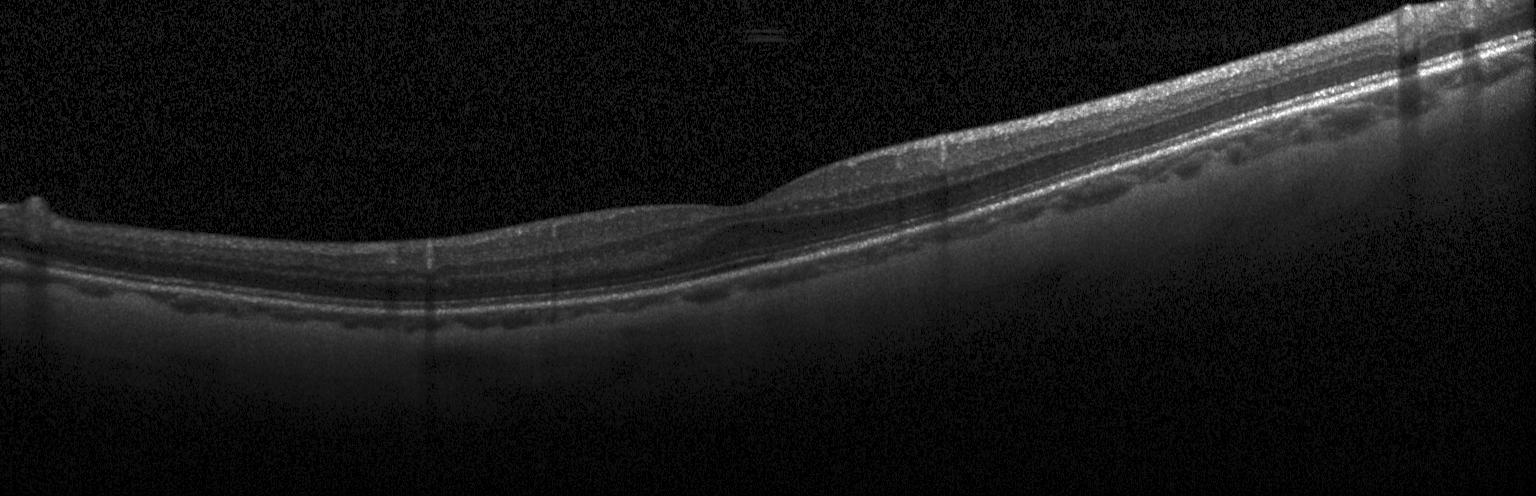 SD-OCT · retinal OCT B-scan.
Finding: no choroidal neovascularization, diabetic macular edema, or drusen.